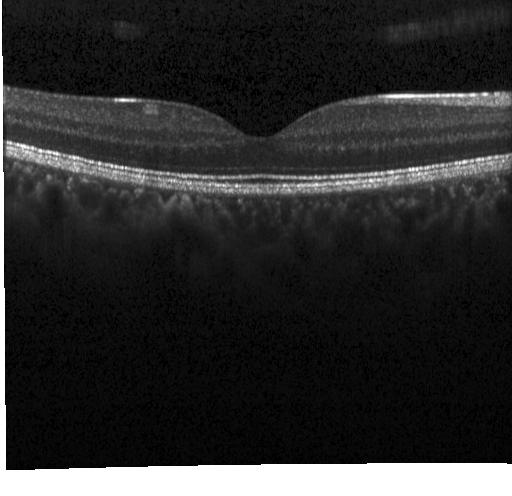

Macular scan; retinal OCT cross-section; Heidelberg Spectralis; spectral-domain optical coherence tomography.
Assessment: no evidence of choroidal neovascularization, diabetic macular edema, or drusen.